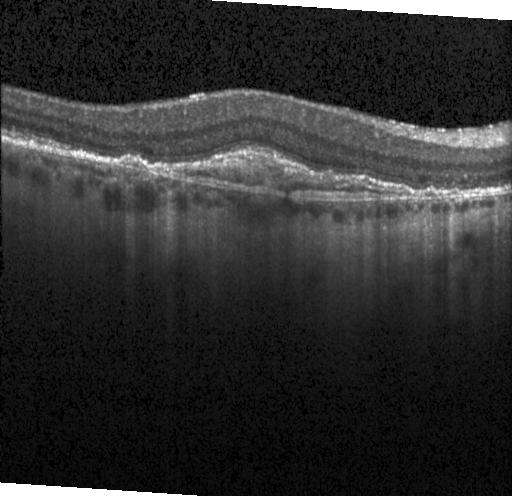 Fovea-centered, spectral-domain OCT, optical coherence tomography scan. Finding: a choroidal neovascular membrane.